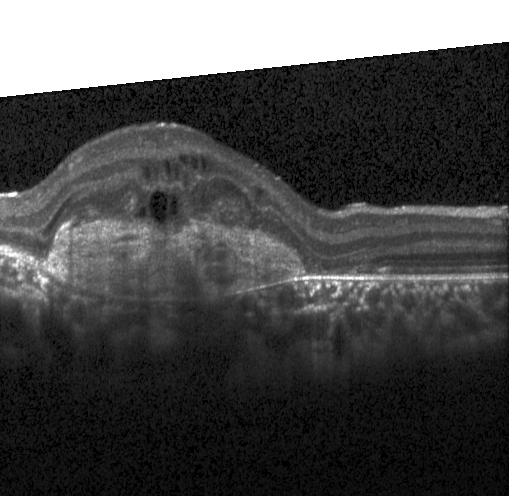

Heidelberg Spectralis OCT system. Retinal OCT cross-section. Finding: a choroidal neovascular membrane.